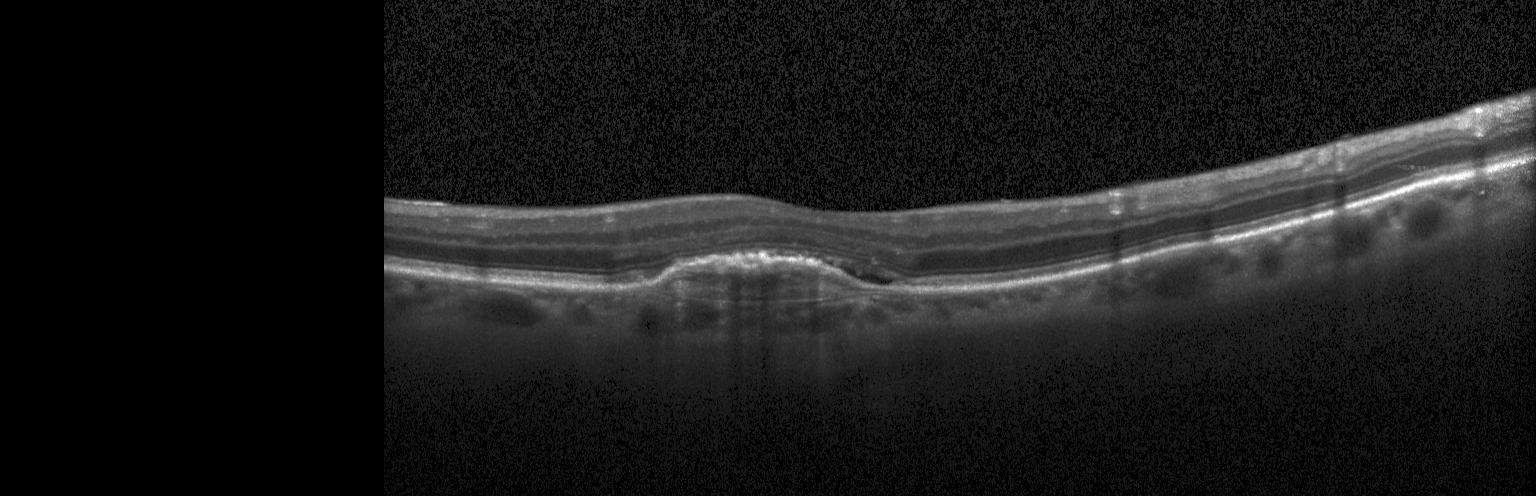 SD-OCT · through the macula · retinal OCT B-scan · instrument: Heidelberg Spectralis. The scan shows choroidal neovascularization.